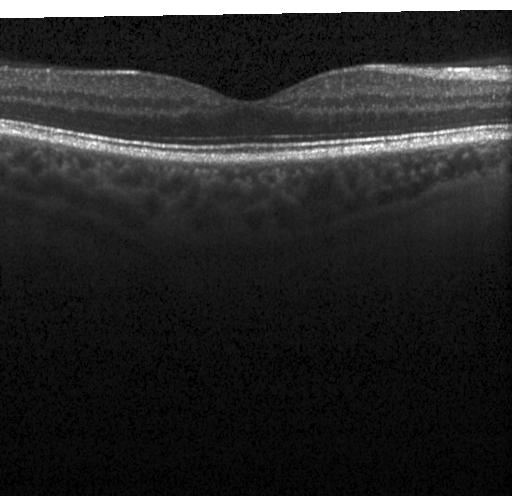 Heidelberg Spectralis OCT system; retinal OCT cross-section — No choroidal neovascularization, no diabetic macular edema, and no drusen.